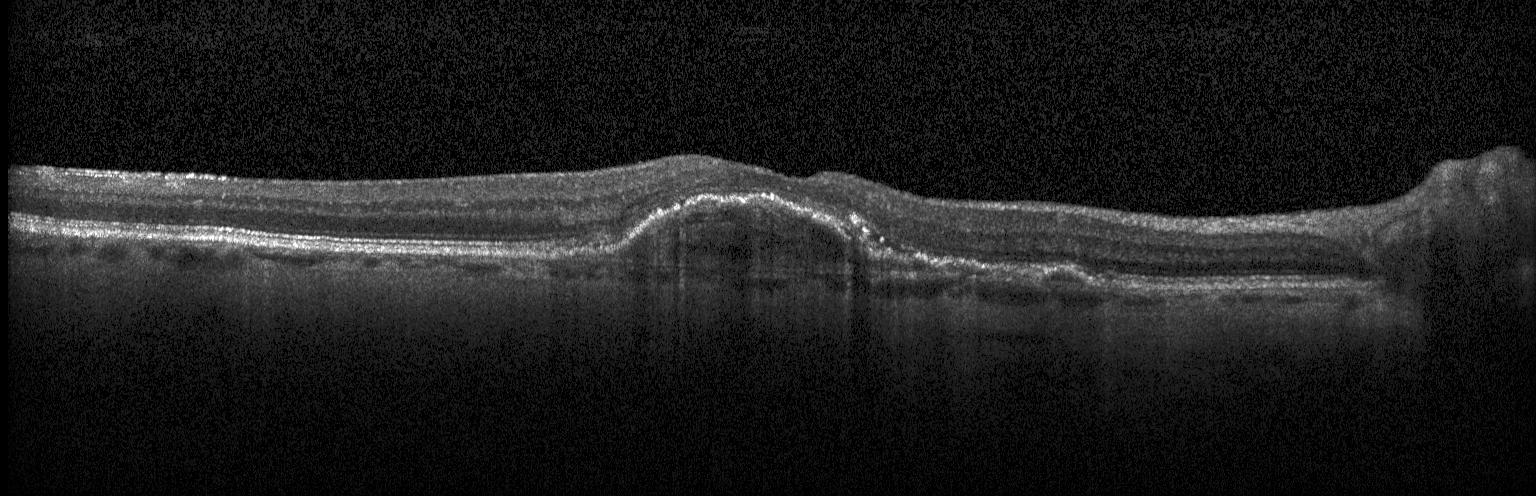
Retinal OCT cross-section showing a choroidal neovascular membrane.